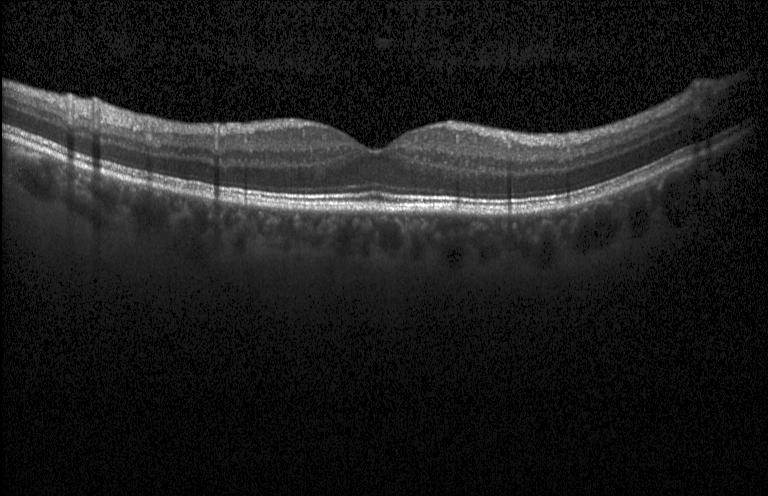
Optical coherence tomography scan, centered on the fovea, Heidelberg Spectralis OCT system, spectral-domain OCT
Finding: neither CNV, DME, nor drusen.